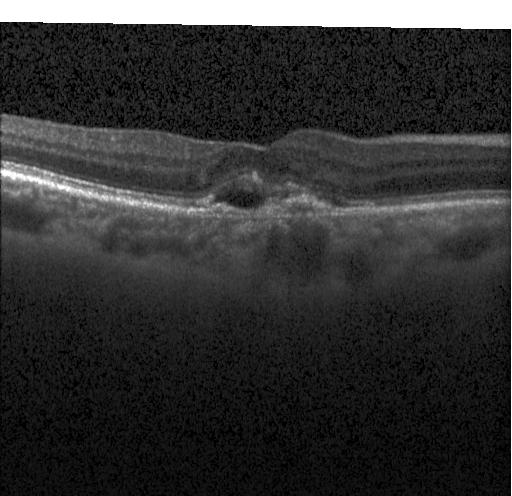
Heidelberg Spectralis · spectral-domain optical coherence tomography · OCT line scan — Finding: choroidal neovascularization.